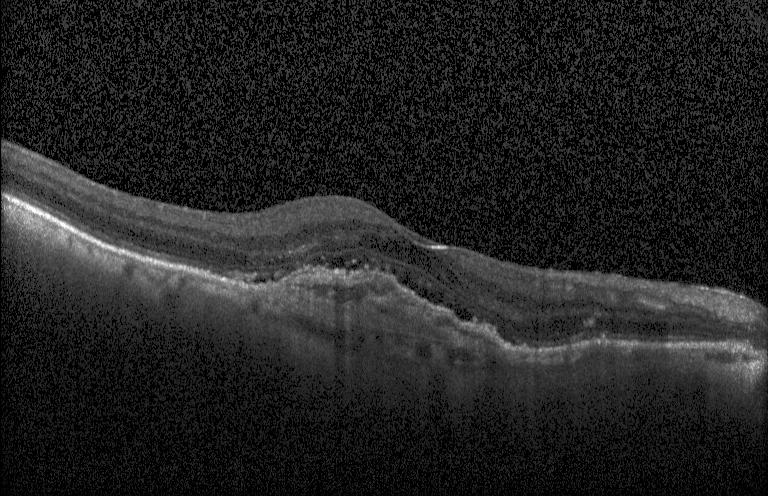 Optical coherence tomography B-scan. Heidelberg Spectralis OCT system — Finding: a choroidal neovascular membrane.